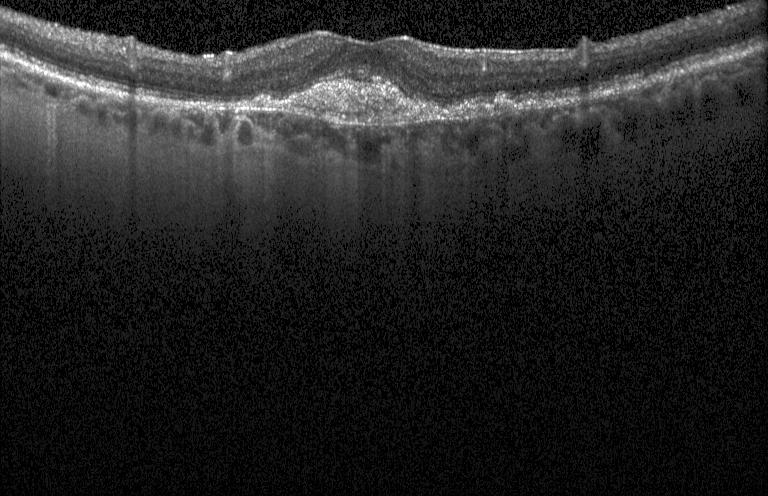

OCT B-scan — Macular OCT: a choroidal neovascular membrane.